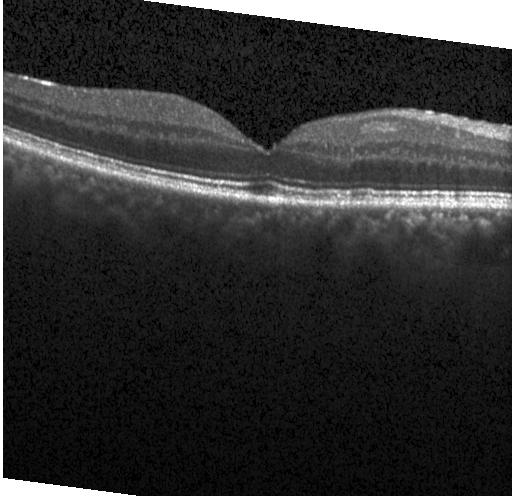 Spectral-domain OCT, OCT B-scan, acquired on a Heidelberg Spectralis, through the macula.
Impression: no evidence of choroidal neovascularization, diabetic macular edema, or drusen.